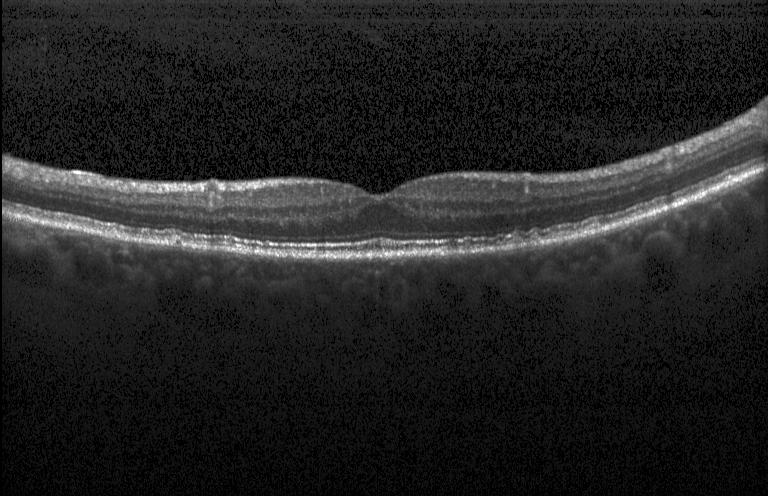 Impression: sub-RPE drusenoid deposits.